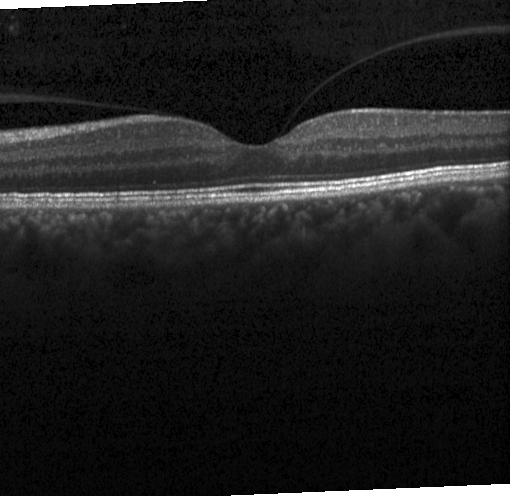
Dx: no CNV, no DME, and no drusen.